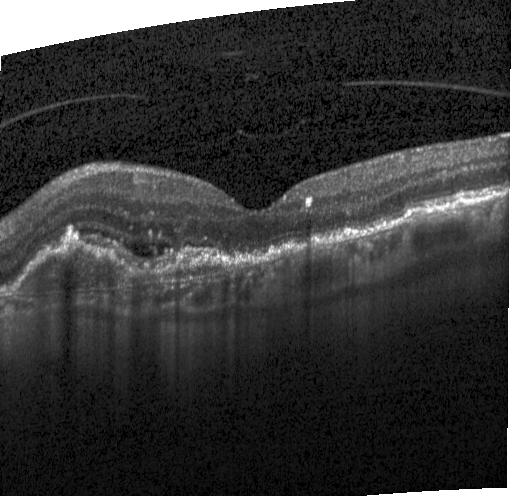
Acquired on a Heidelberg Spectralis, through the macula, optical coherence tomography B-scan. Finding: choroidal neovascularization.